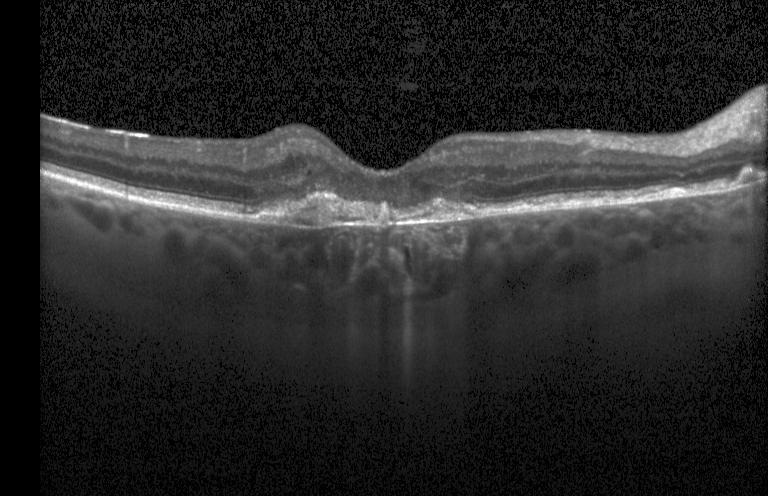
Macular OCT demonstrating CNV.